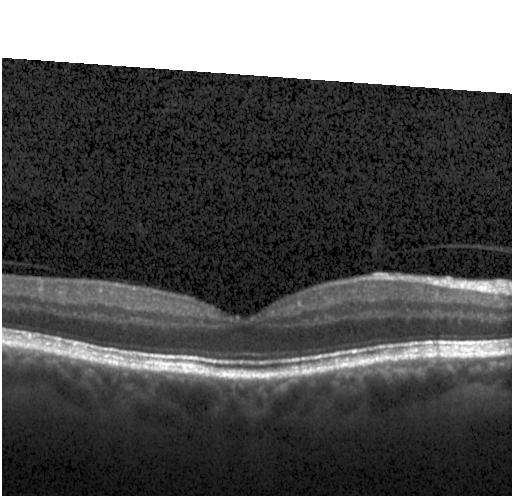

Spectral-domain OCT B-scan: no choroidal neovascularization, no diabetic macular edema, and no drusen.